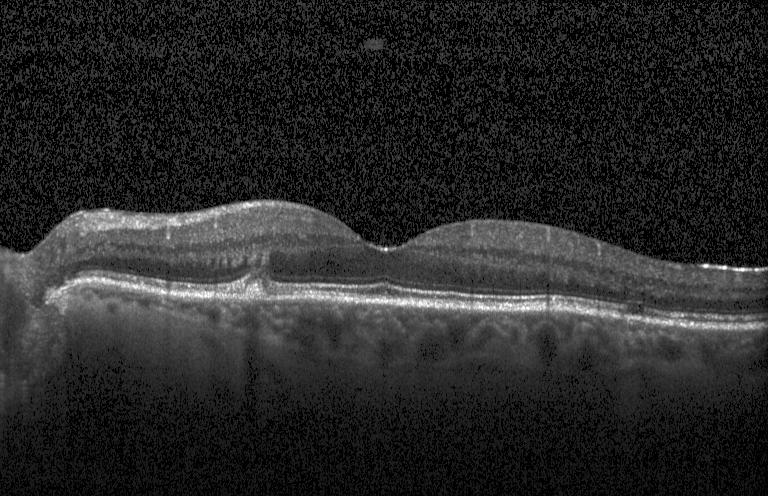 Macular OCT: multiple drusen.